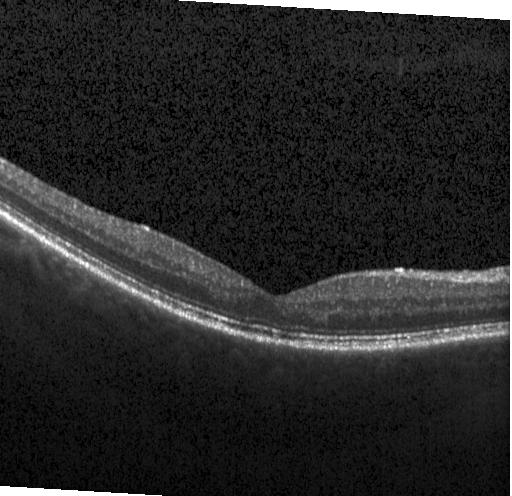
OCT scan showing neither choroidal neovascularization, diabetic macular edema, nor drusen.